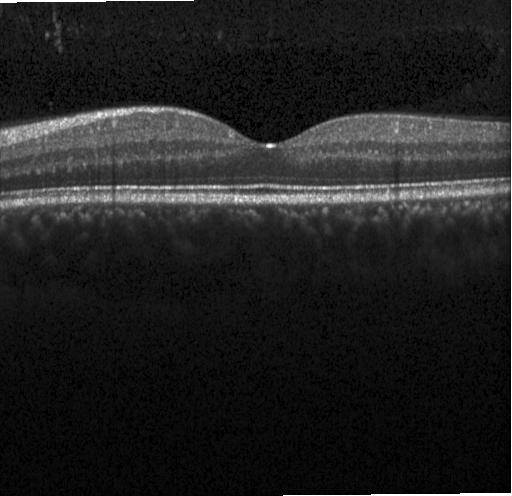
Spectral-domain OCT; optical coherence tomography B-scan; macular scan
Macular OCT: no evidence of choroidal neovascularization, diabetic macular edema, or drusen.